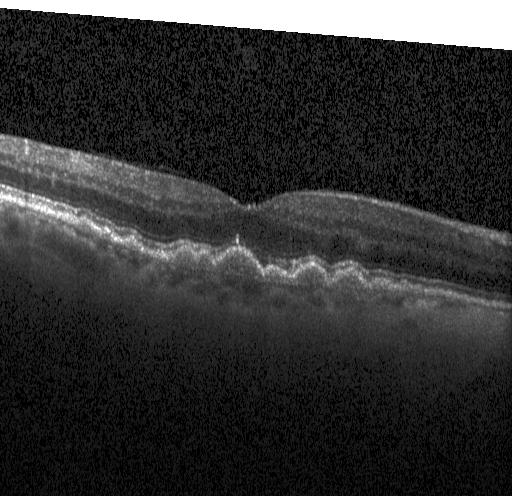
Optical coherence tomography B-scan.
Diagnosis: sub-RPE drusenoid deposits.